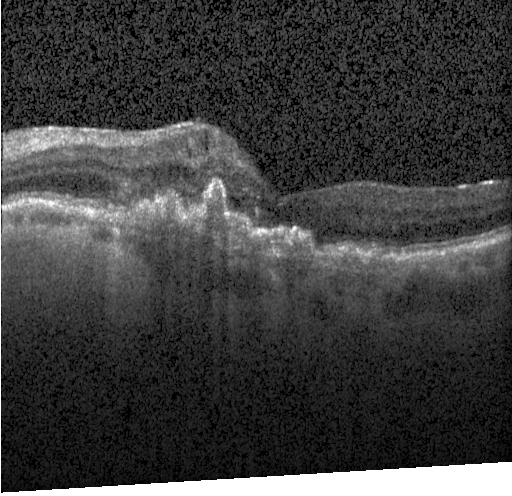
OCT finding: CNV.